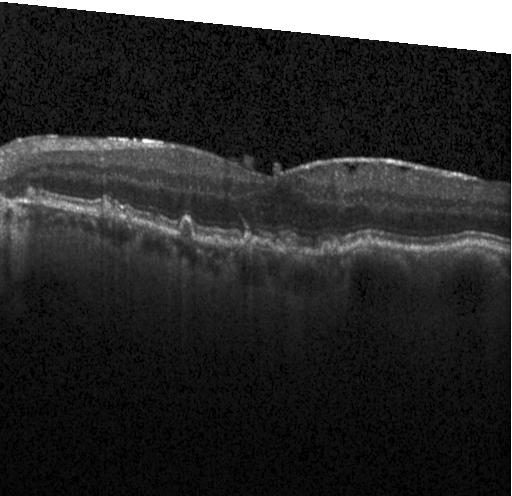 Assessment: sub-RPE drusenoid deposits.